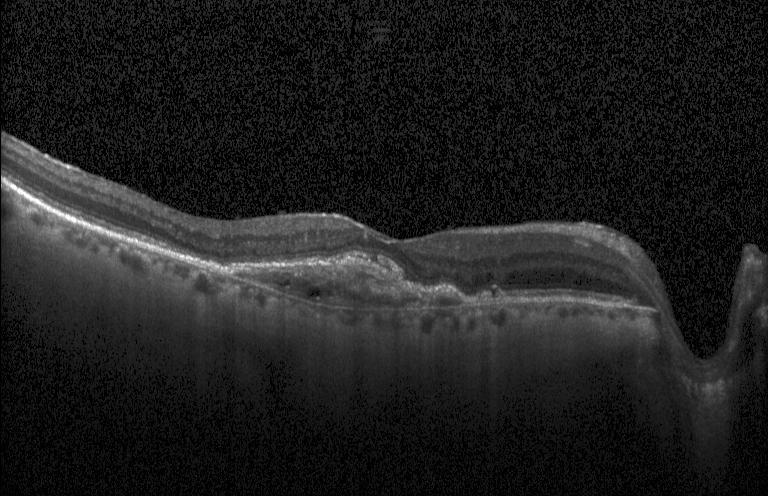
Spectral-domain optical coherence tomography, horizontal scan through the fovea, retinal OCT B-scan, Heidelberg Spectralis. Impression: a choroidal neovascular membrane.